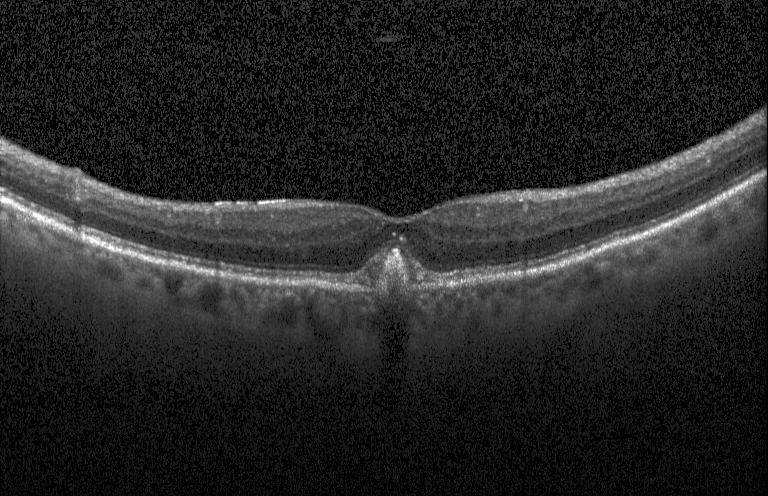

Diagnosis: a choroidal neovascular membrane.